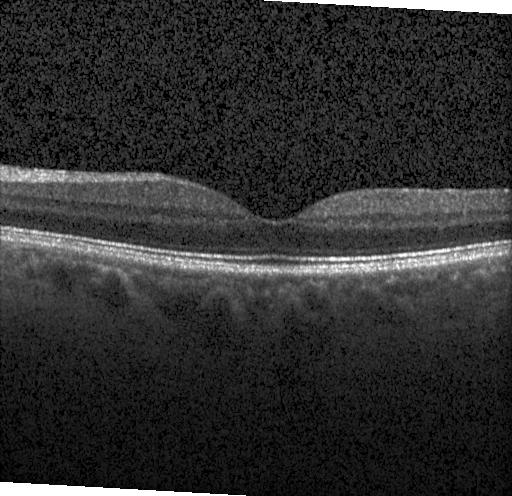 Through the macula, optical coherence tomography B-scan, spectral-domain optical coherence tomography — Finding: neither choroidal neovascularization, diabetic macular edema, nor drusen.